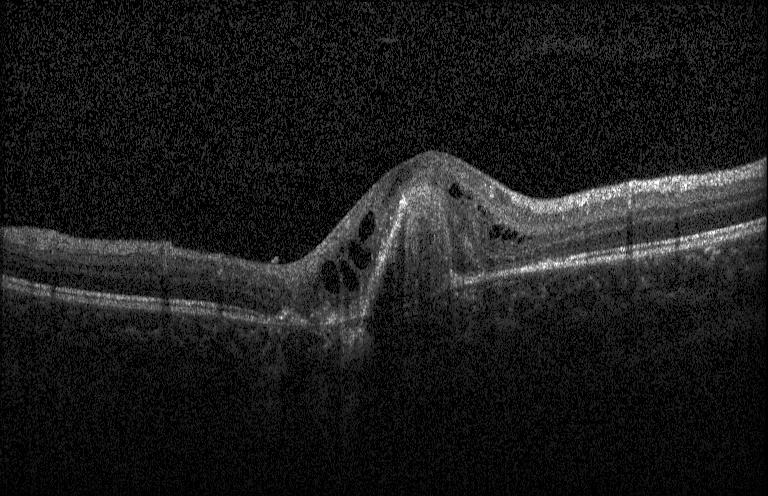 The scan shows choroidal neovascularization (CNV).